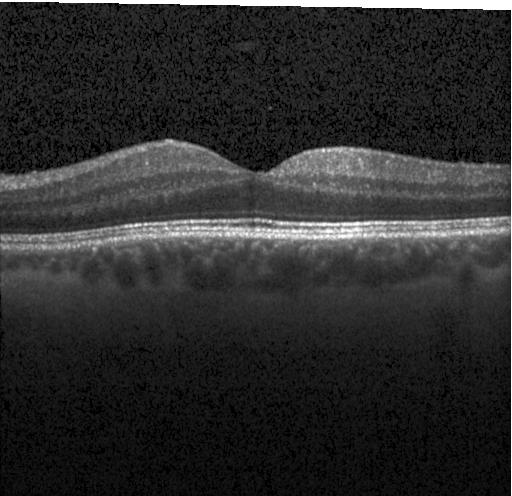
OCT scan showing no evidence of choroidal neovascularization, diabetic macular edema, or drusen.